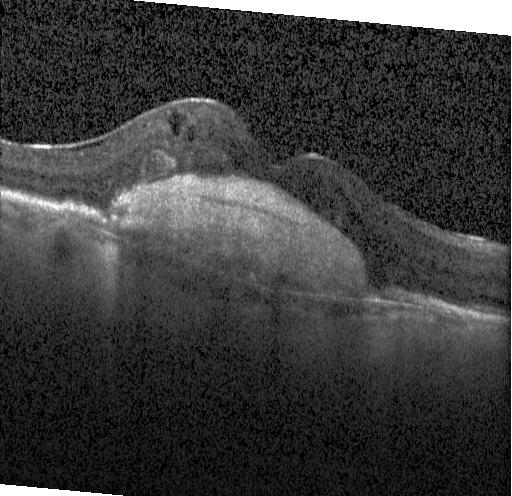

Spectral-domain OCT B-scan: choroidal neovascularization (CNV).